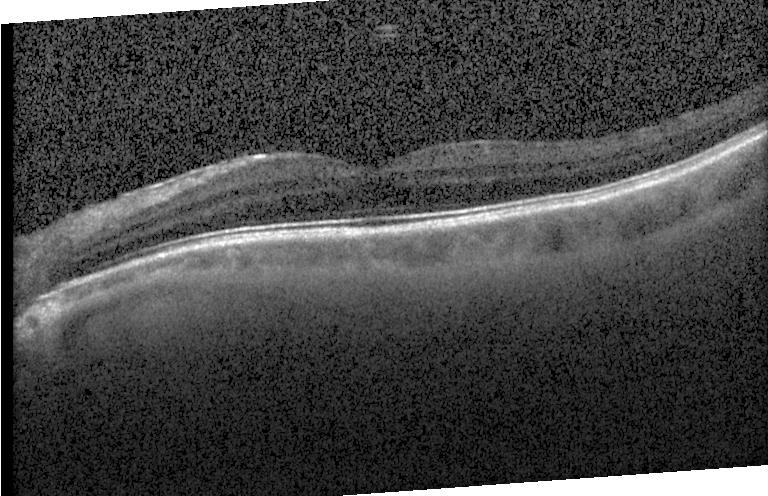

Fovea-centered; spectral-domain optical coherence tomography; optical coherence tomography B-scan. Assessment: no CNV, no DME, and no drusen.